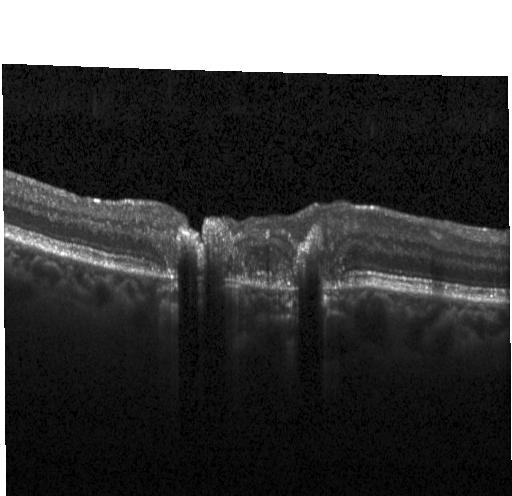
OCT finding: a choroidal neovascular membrane.